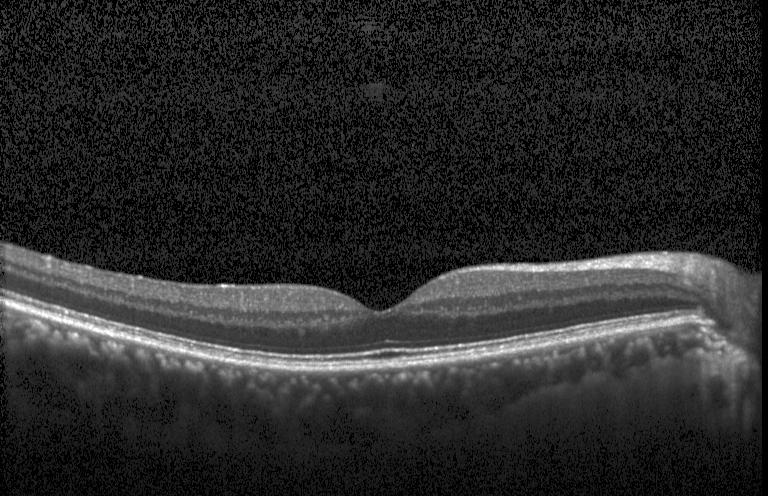

Assessment: neither CNV, DME, nor drusen.